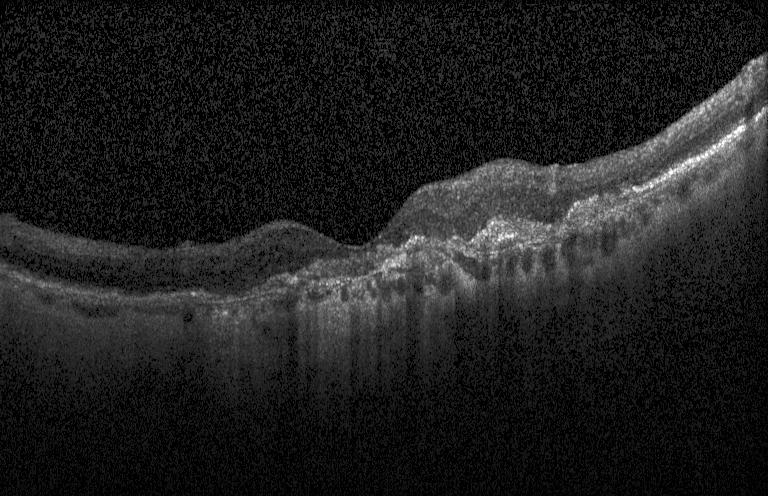

SD-OCT. Optical coherence tomography B-scan — Finding: a choroidal neovascular membrane.